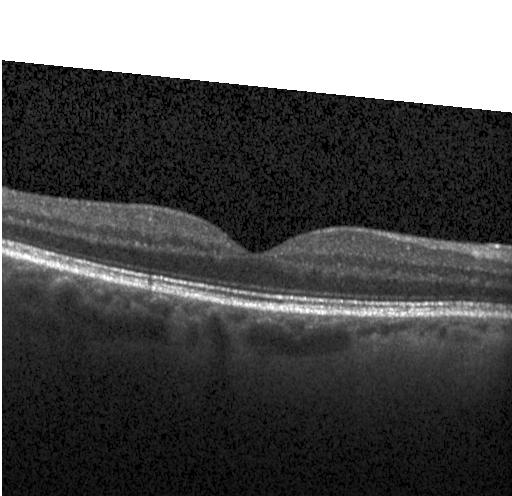
OCT finding: no choroidal neovascularization, no diabetic macular edema, and no drusen.